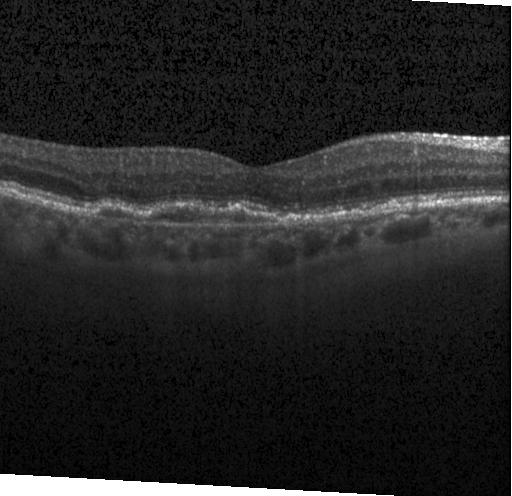

Retinal OCT B-scan — The scan shows a choroidal neovascular membrane.